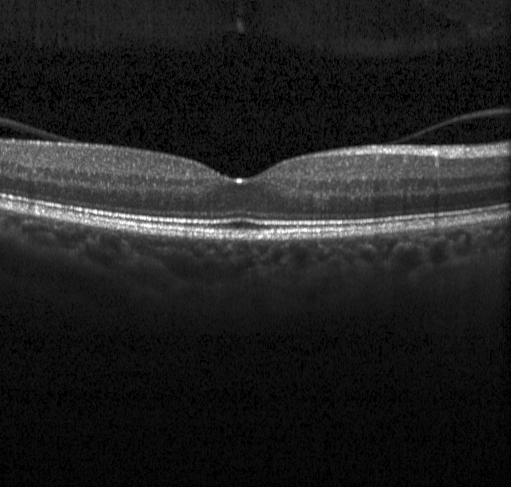 Impression: no evidence of choroidal neovascularization, diabetic macular edema, or drusen.